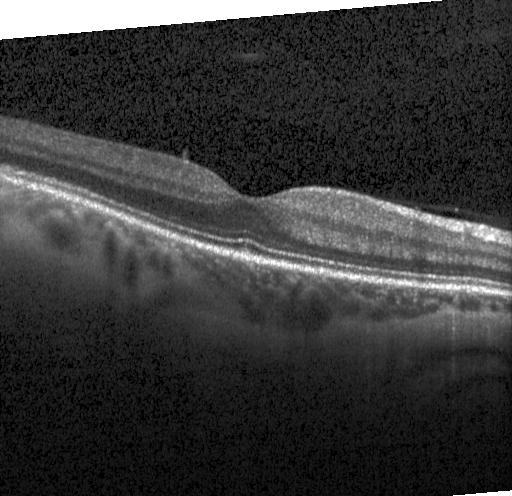 Diagnosis: no evidence of choroidal neovascularization, diabetic macular edema, or drusen.